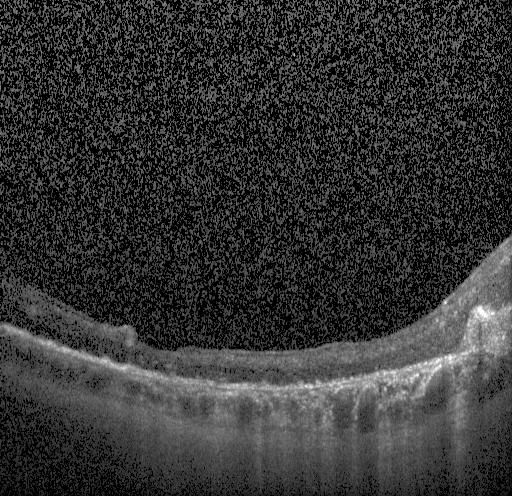 Macular OCT demonstrating CNV.